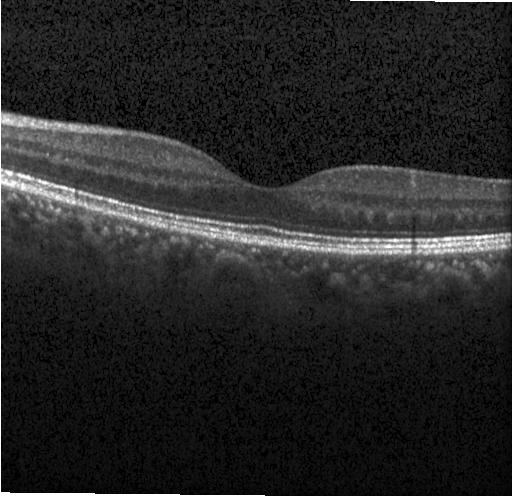
Diagnosis: neither CNV, DME, nor drusen.